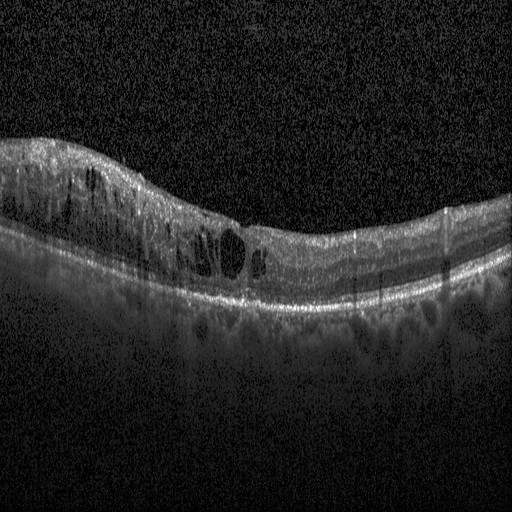
Diagnosis: diabetic macular edema (DME).